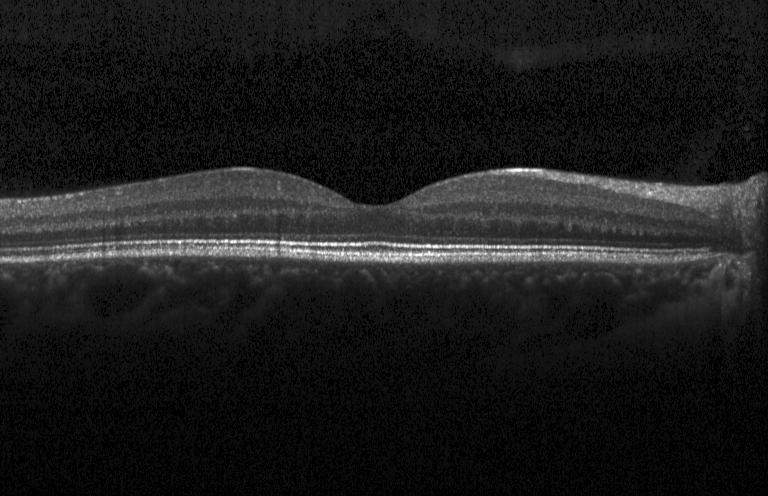
Fovea-centered; Heidelberg Spectralis OCT system; spectral-domain OCT; optical coherence tomography scan.
Impression: no choroidal neovascularization, diabetic macular edema, or drusen.